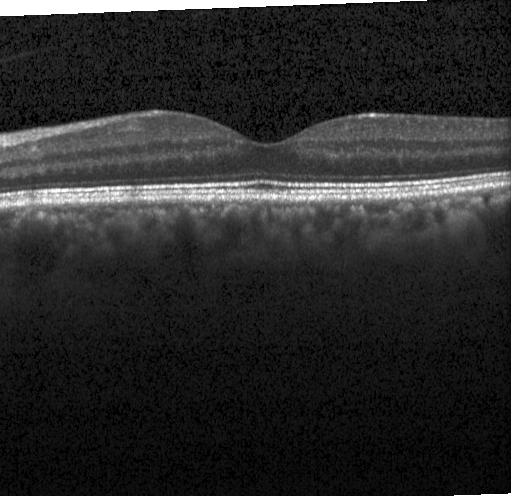
Spectral-domain optical coherence tomography · acquired on a Heidelberg Spectralis · centered on the fovea · retinal OCT B-scan. Finding: neither choroidal neovascularization, diabetic macular edema, nor drusen.